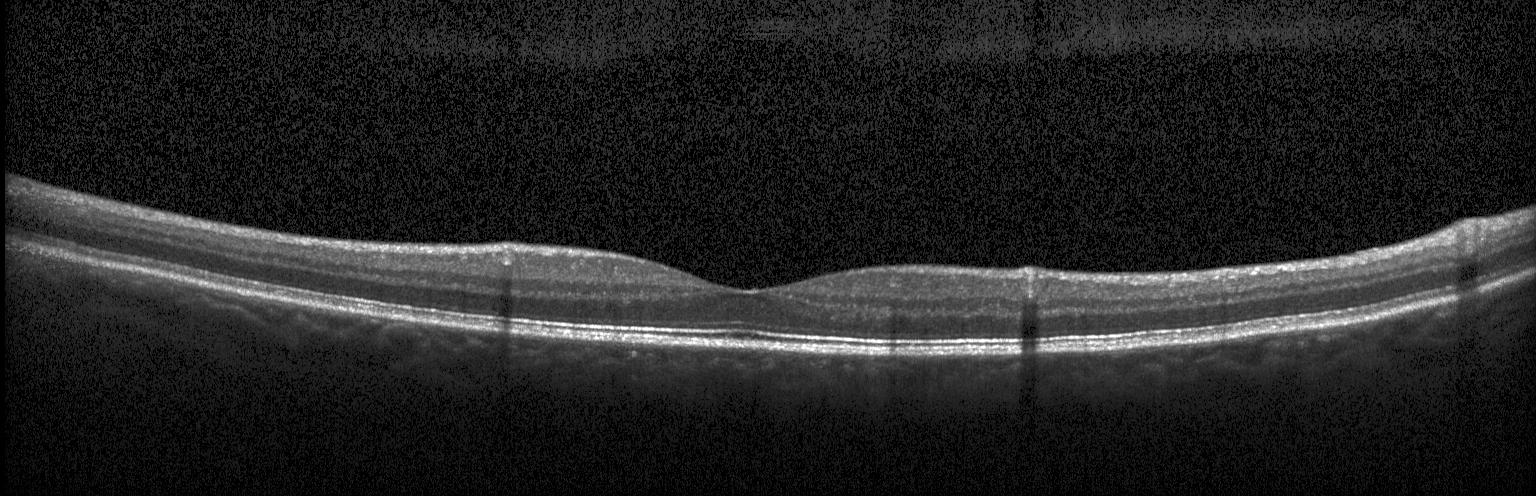 Spectral-domain OCT, fovea-centered, OCT B-scan, Heidelberg Spectralis.
Dx: no choroidal neovascularization, diabetic macular edema, or drusen.